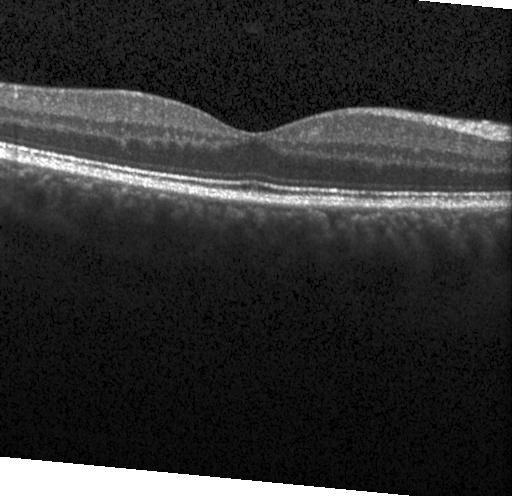

Acquired on a Heidelberg Spectralis. OCT B-scan — Finding: no choroidal neovascularization, diabetic macular edema, or drusen.